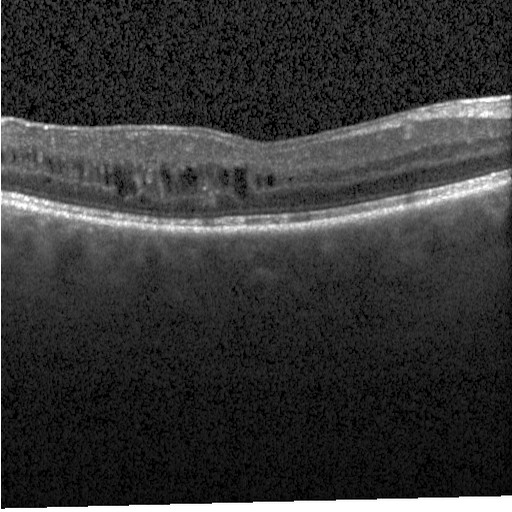
Centered on the fovea. SD-OCT. Optical coherence tomography scan. Heidelberg Spectralis OCT system — Diagnosis: diabetic macular edema.